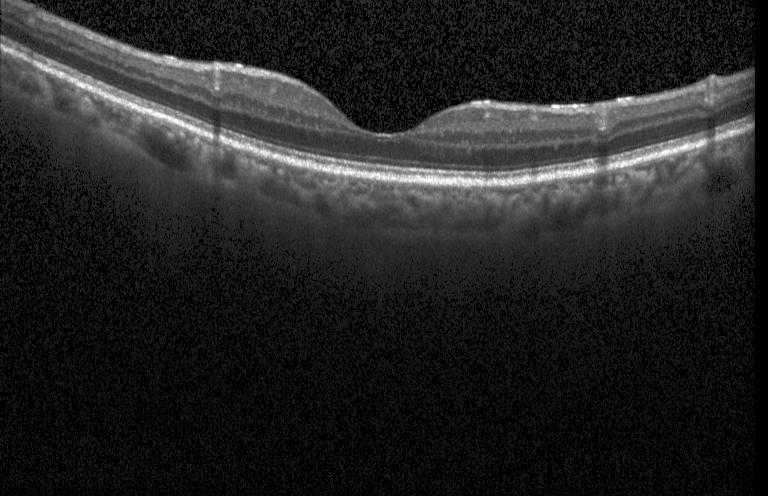
The scan shows no choroidal neovascularization, diabetic macular edema, or drusen.